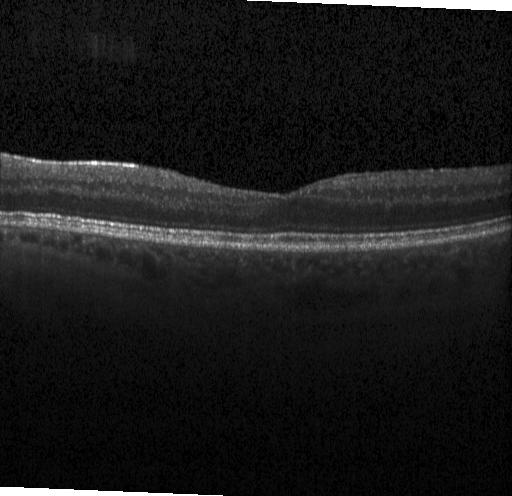

Fovea-centered · optical coherence tomography scan
The scan shows neither CNV, DME, nor drusen.